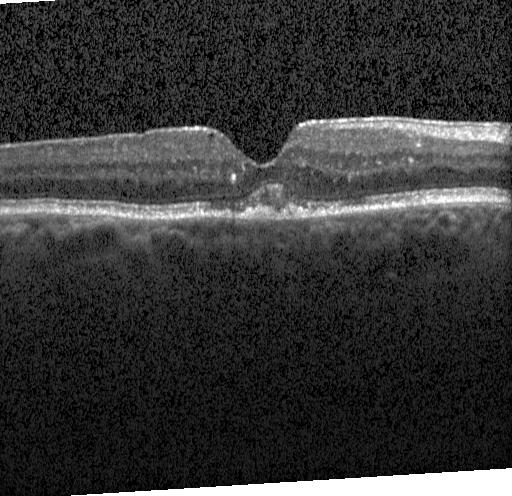 Diagnosis: a choroidal neovascular membrane.